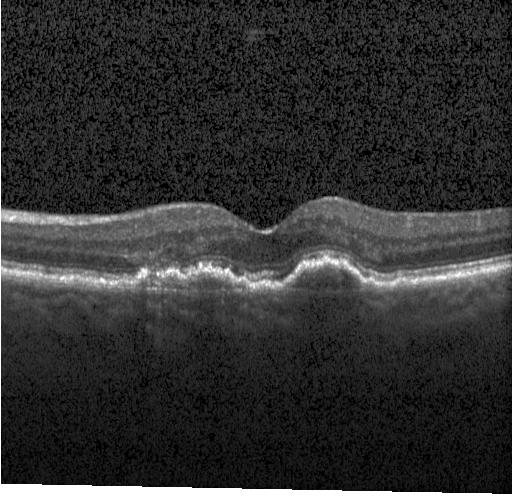
Retinal OCT B-scan; SD-OCT; acquired on a Heidelberg Spectralis; centered on the fovea
The scan shows choroidal neovascularization.